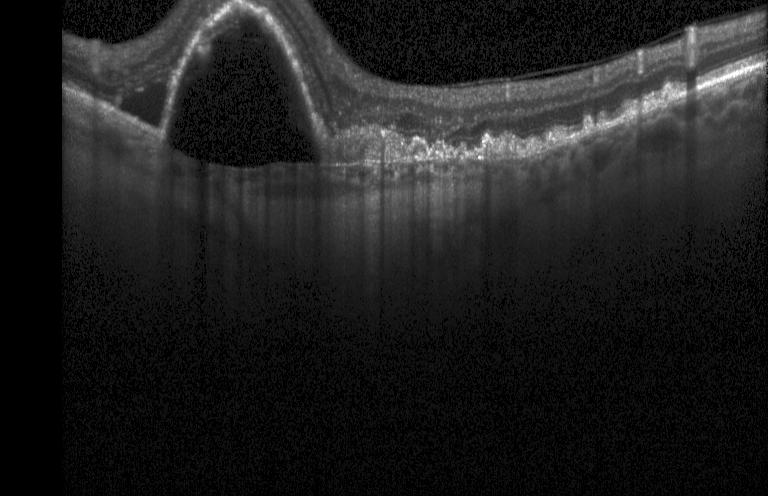

Diagnosis: choroidal neovascularization.